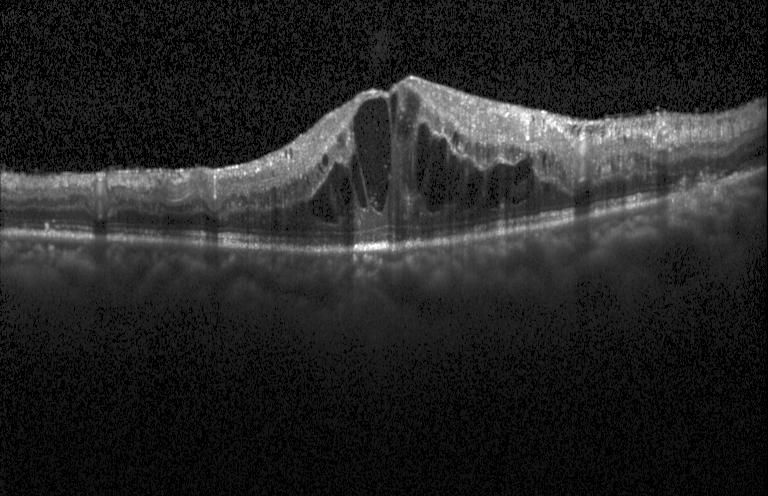 Retinal OCT B-scan. Spectral-domain OCT. Finding: DME.